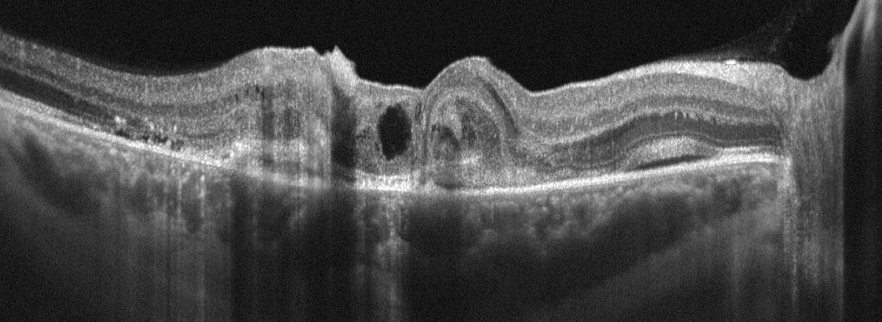
Retinal OCT B-scan. Oculus dexter — Macular OCT: age-related macular degeneration (AMD).